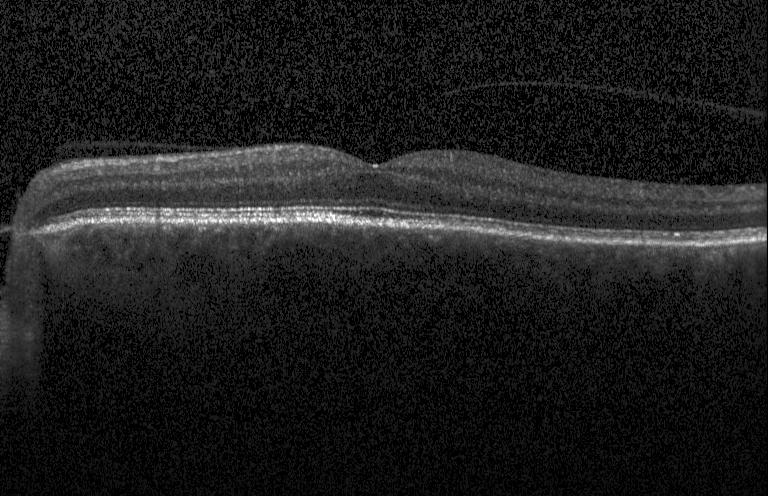 Diagnosis: no evidence of CNV, DME, or drusen.